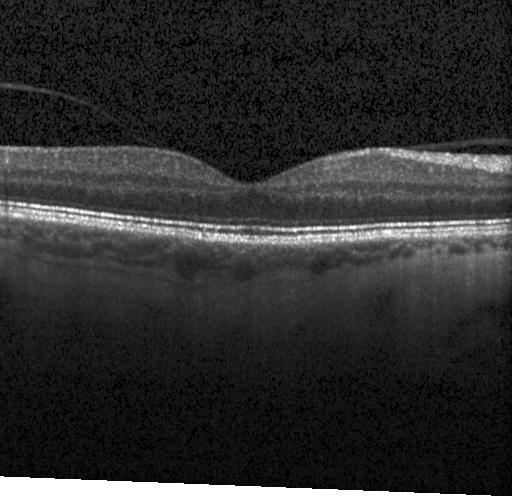
OCT B-scan, Heidelberg Spectralis OCT system, centered on the fovea — Impression: no choroidal neovascularization, no diabetic macular edema, and no drusen.